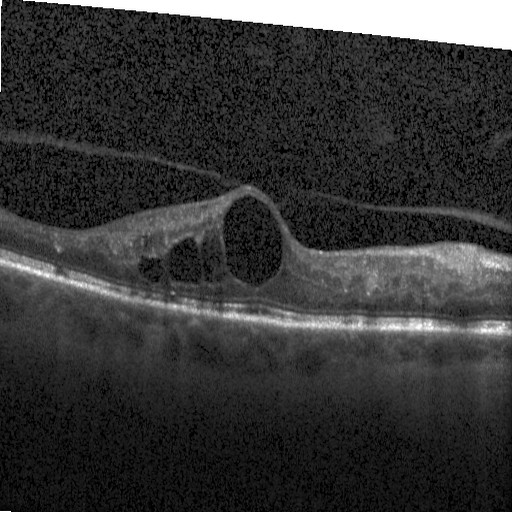 Retinal OCT cross-section. Fovea-centered. Finding: diabetic macular edema.